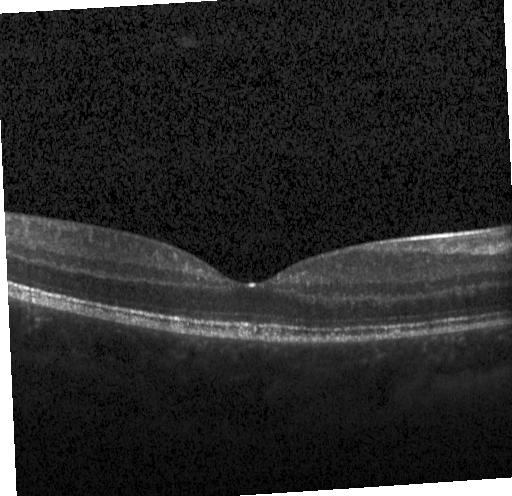

OCT B-scan showing no evidence of choroidal neovascularization, diabetic macular edema, or drusen.